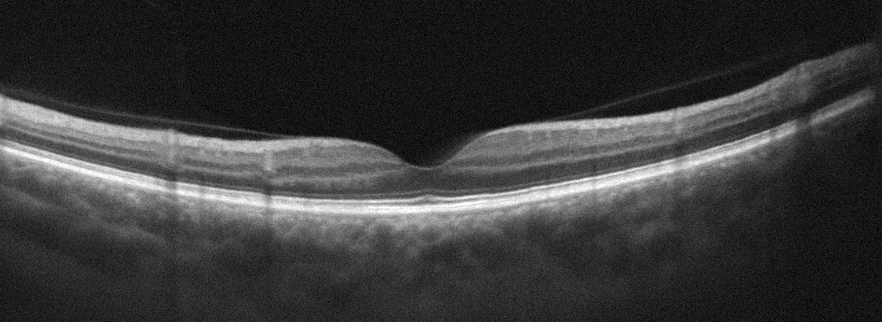
Oculus dexter; OCT B-scan — Finding: no AMD, DME, ERM, RAO, RVO, or VID.